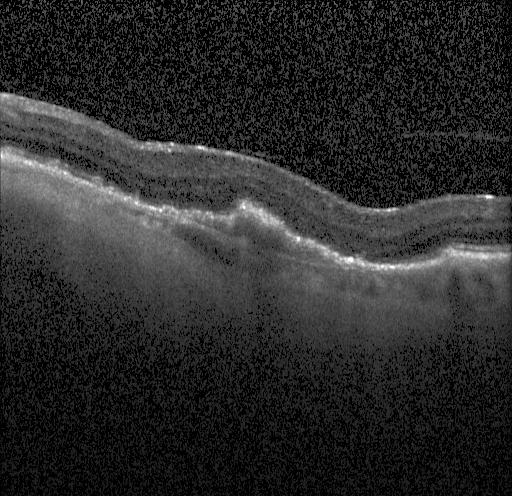 Spectral-domain OCT, OCT line scan.
This B-scan demonstrates a choroidal neovascular membrane.